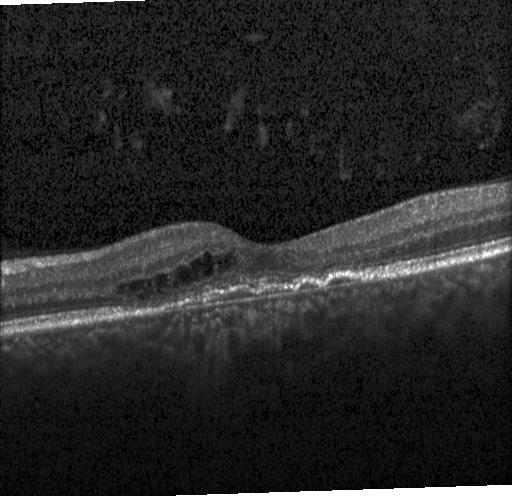

OCT B-scan showing CNV.